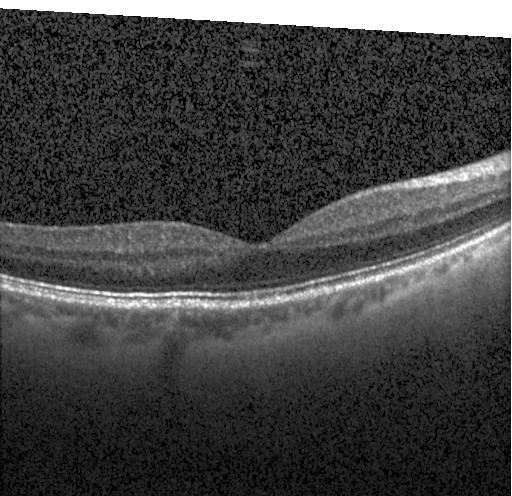 OCT B-scan. Through the macula. Heidelberg Spectralis OCT system. SD-OCT. Diagnosis: no evidence of choroidal neovascularization, diabetic macular edema, or drusen.